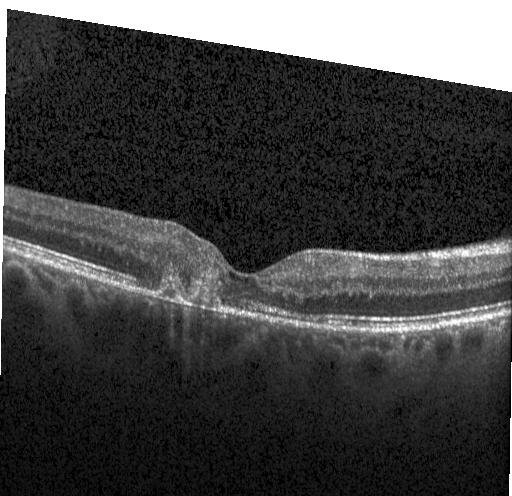 Diagnosis: choroidal neovascularization (CNV).